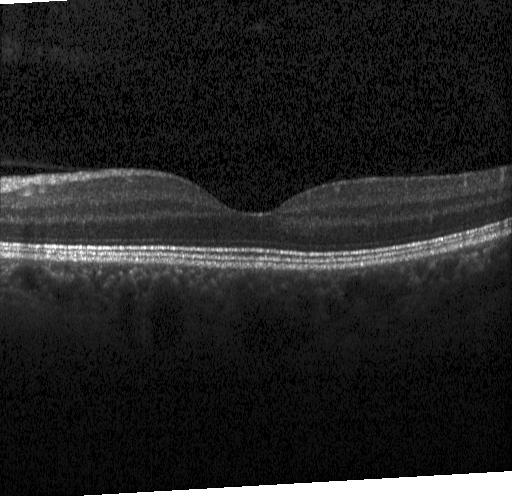
Impression: no choroidal neovascularization, diabetic macular edema, or drusen.